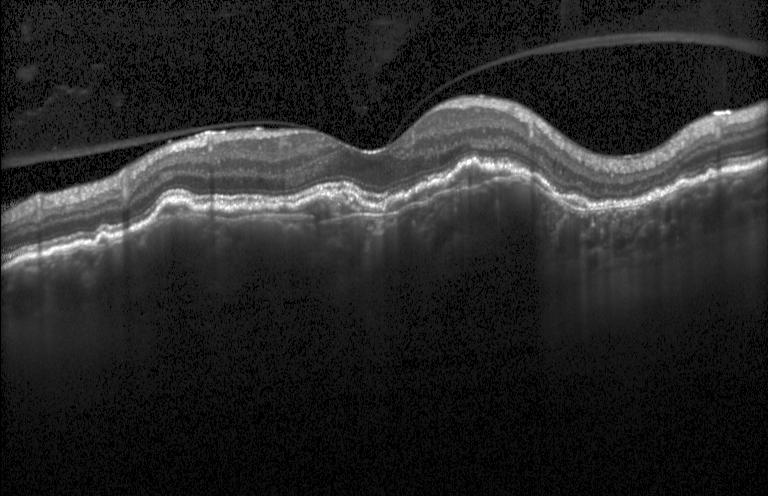
Retinal OCT cross-section showing CNV.